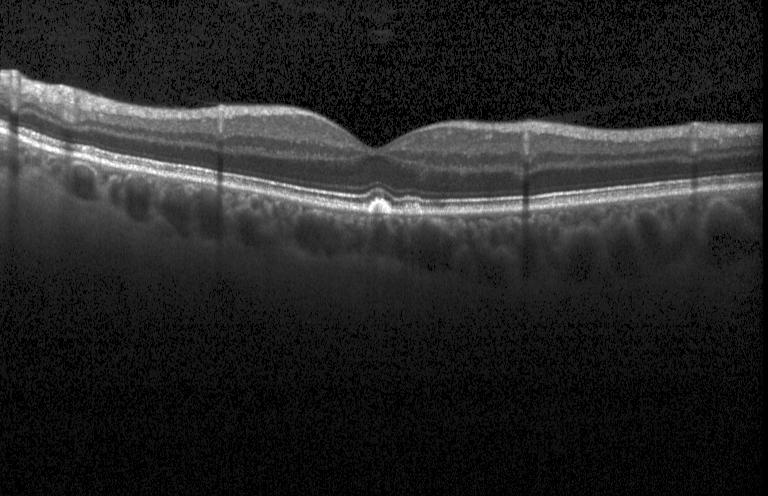
OCT scan showing drusen.